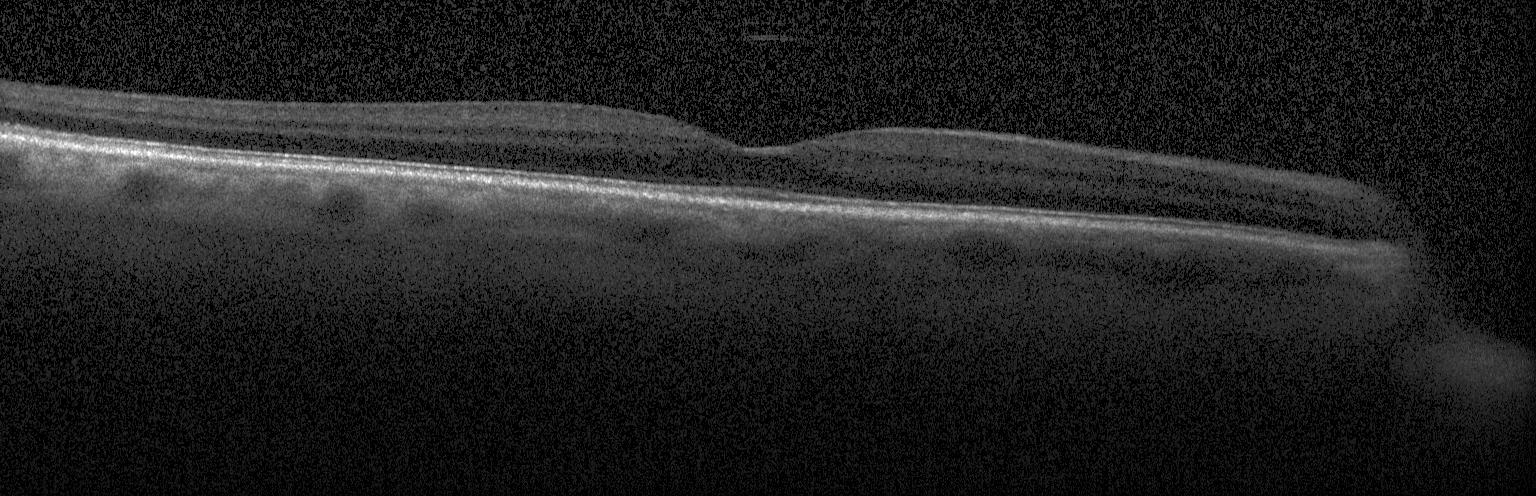 Macular scan, retinal OCT cross-section. Impression: no choroidal neovascularization, no diabetic macular edema, and no drusen.